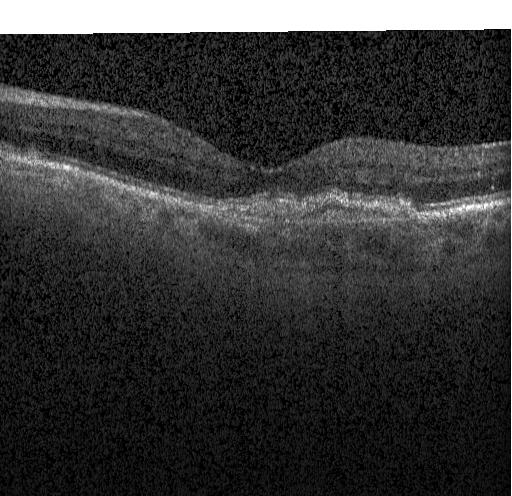 Horizontal scan through the fovea. Spectral-domain optical coherence tomography. Acquired on a Heidelberg Spectralis. Optical coherence tomography B-scan
Dx: choroidal neovascularization.